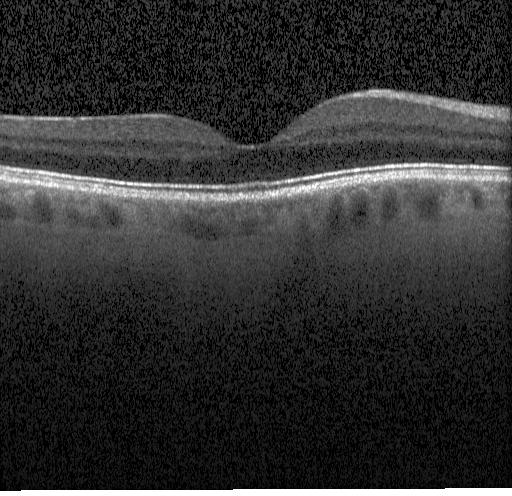

Impression: no CNV, DME, or drusen.